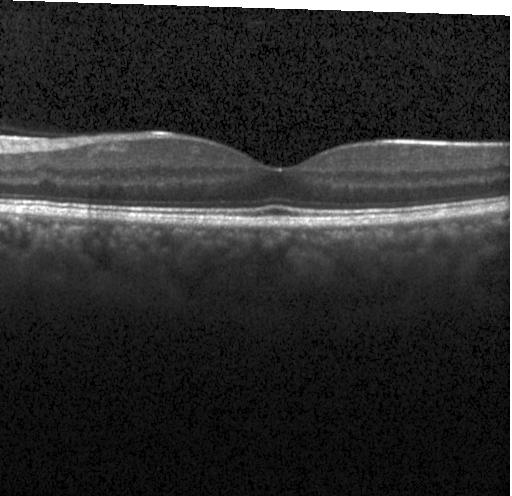 Macular OCT: no evidence of choroidal neovascularization, diabetic macular edema, or drusen.